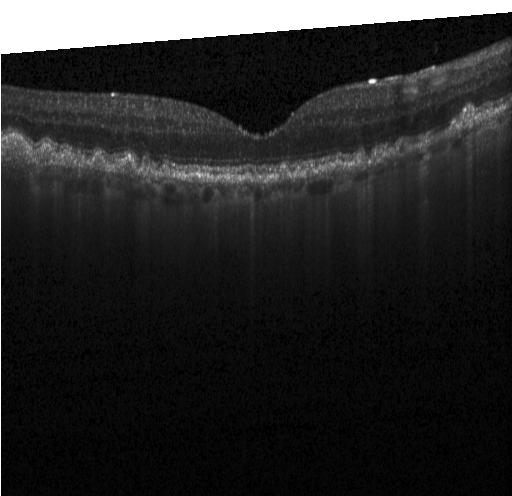

Impression: multiple drusen.